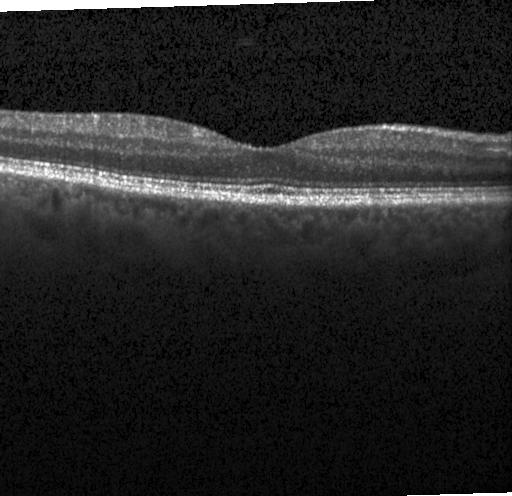 SD-OCT · optical coherence tomography scan.
Macular OCT: no evidence of CNV, DME, or drusen.